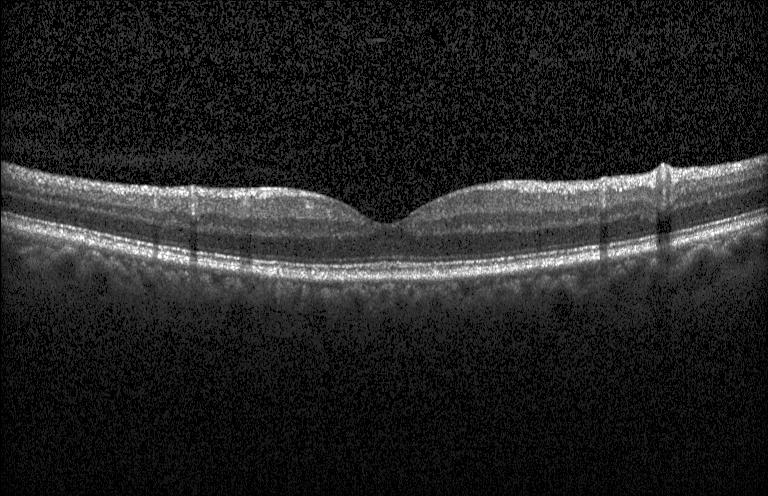

Diagnosis: no choroidal neovascularization, no diabetic macular edema, and no drusen.